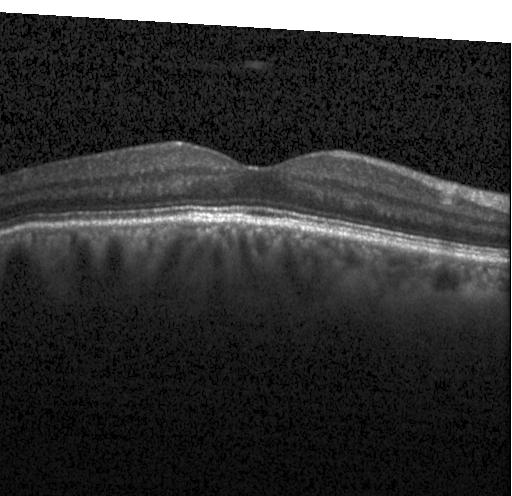

Neither choroidal neovascularization, diabetic macular edema, nor drusen.